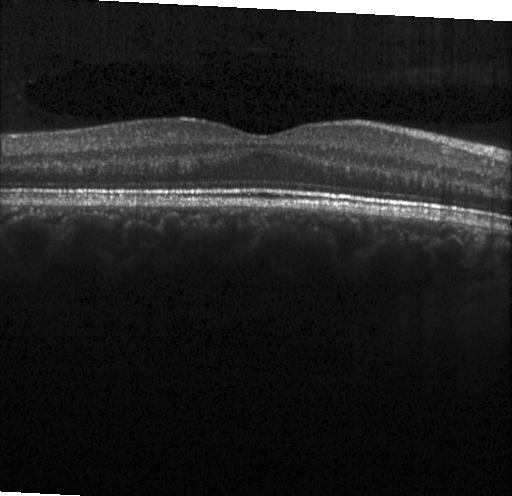 Heidelberg Spectralis. Optical coherence tomography B-scan.
OCT finding: no CNV, DME, or drusen.